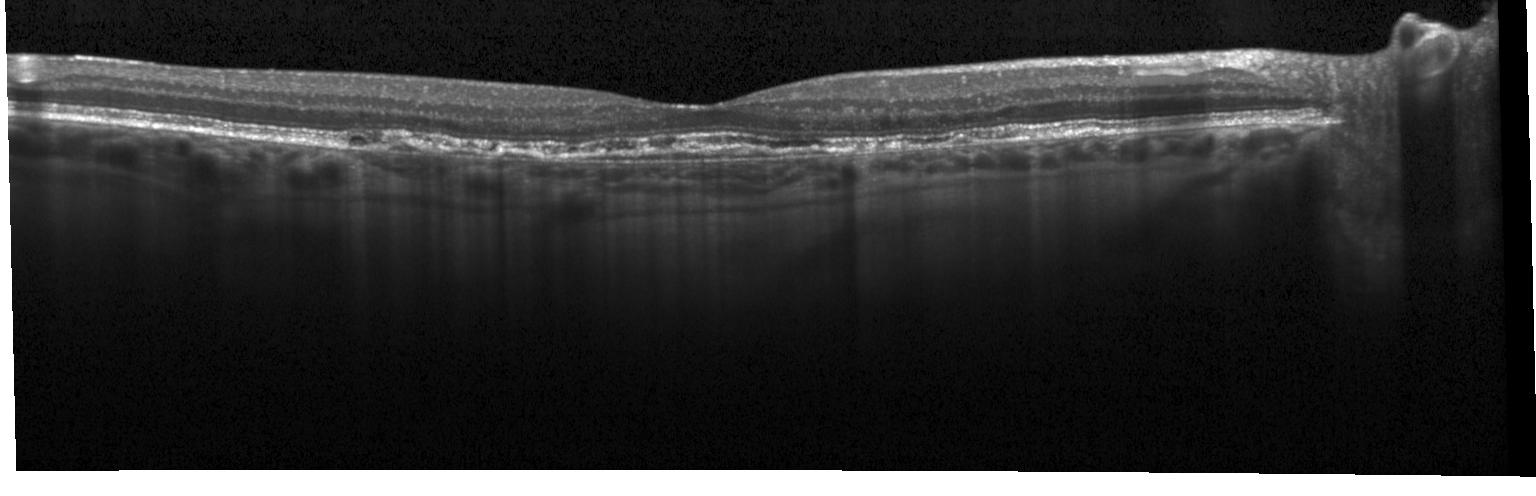
Macular OCT: a choroidal neovascular membrane.